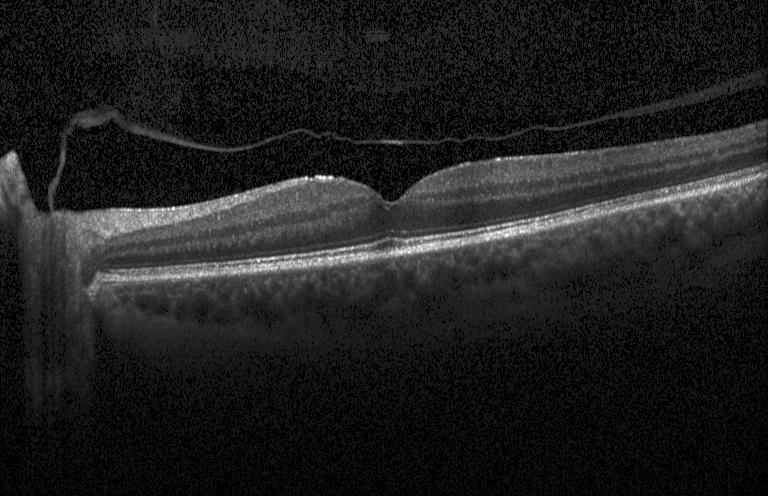
Heidelberg Spectralis. OCT line scan. Horizontal scan through the fovea — Diagnosis: no choroidal neovascularization, diabetic macular edema, or drusen.